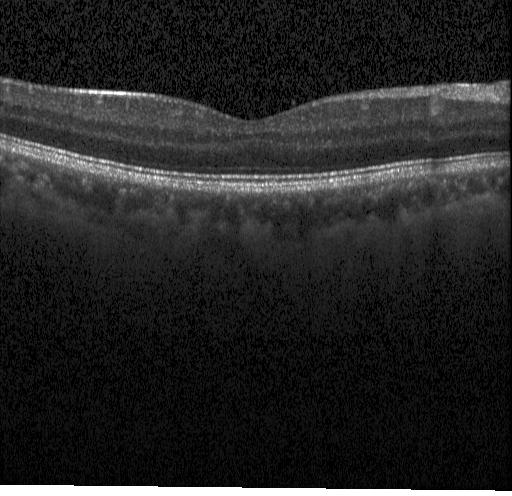
Fovea-centered, spectral-domain optical coherence tomography, Heidelberg Spectralis, optical coherence tomography B-scan. The scan shows neither CNV, DME, nor drusen.